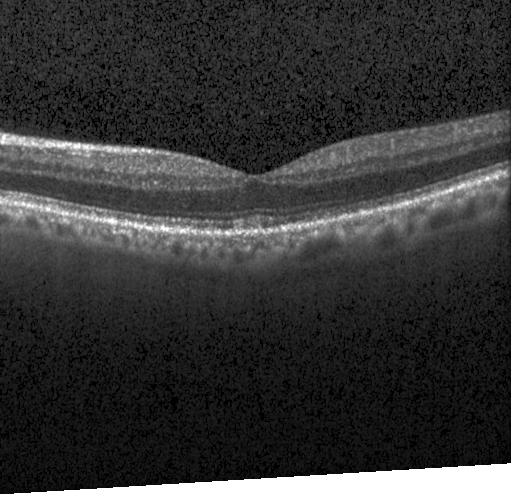 OCT scan showing no evidence of choroidal neovascularization, diabetic macular edema, or drusen.